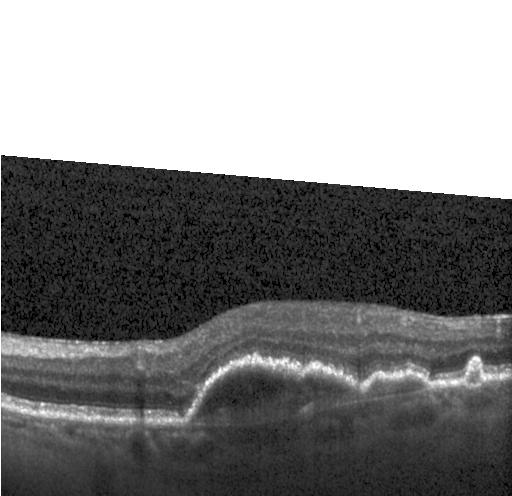

Diagnosis: choroidal neovascularization.